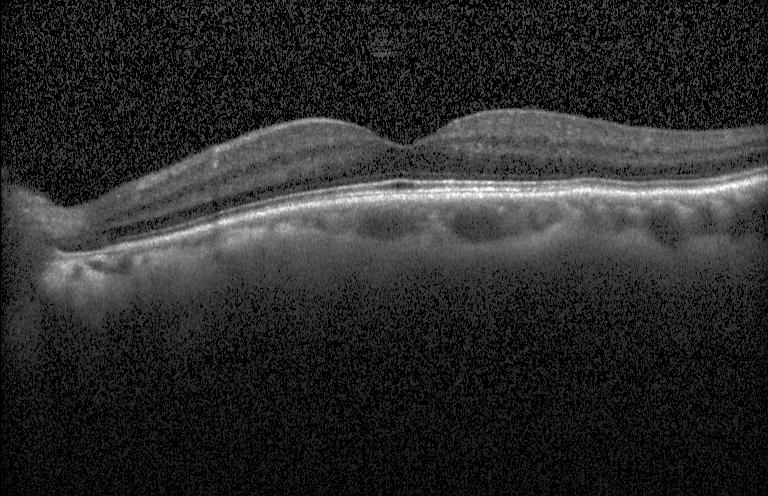

Retinal OCT cross-section showing no choroidal neovascularization, diabetic macular edema, or drusen.